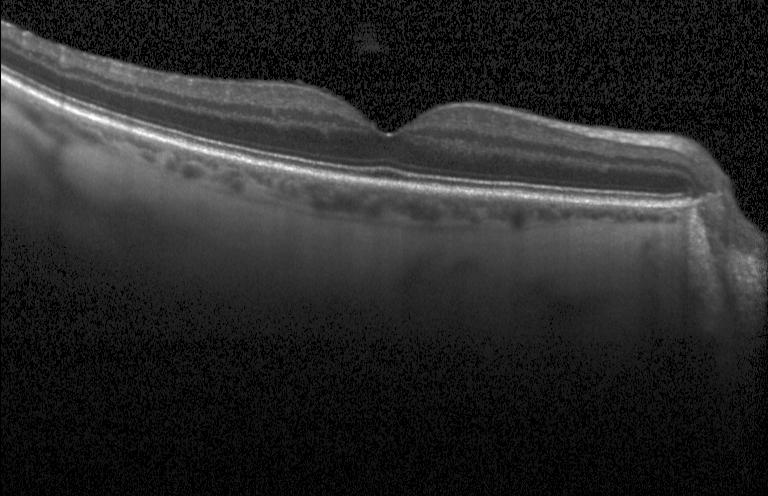 Assessment: neither choroidal neovascularization, diabetic macular edema, nor drusen.